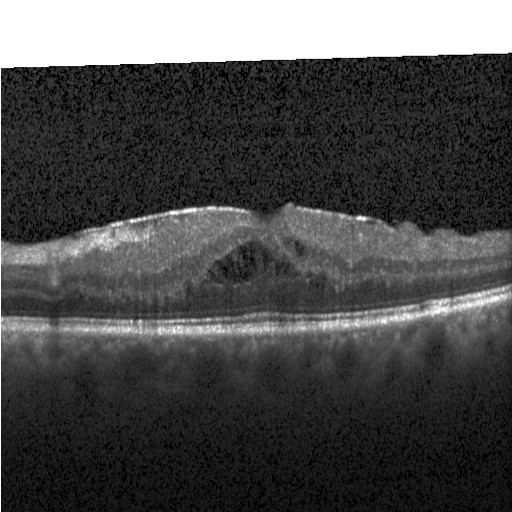
OCT finding: diabetic macular edema.